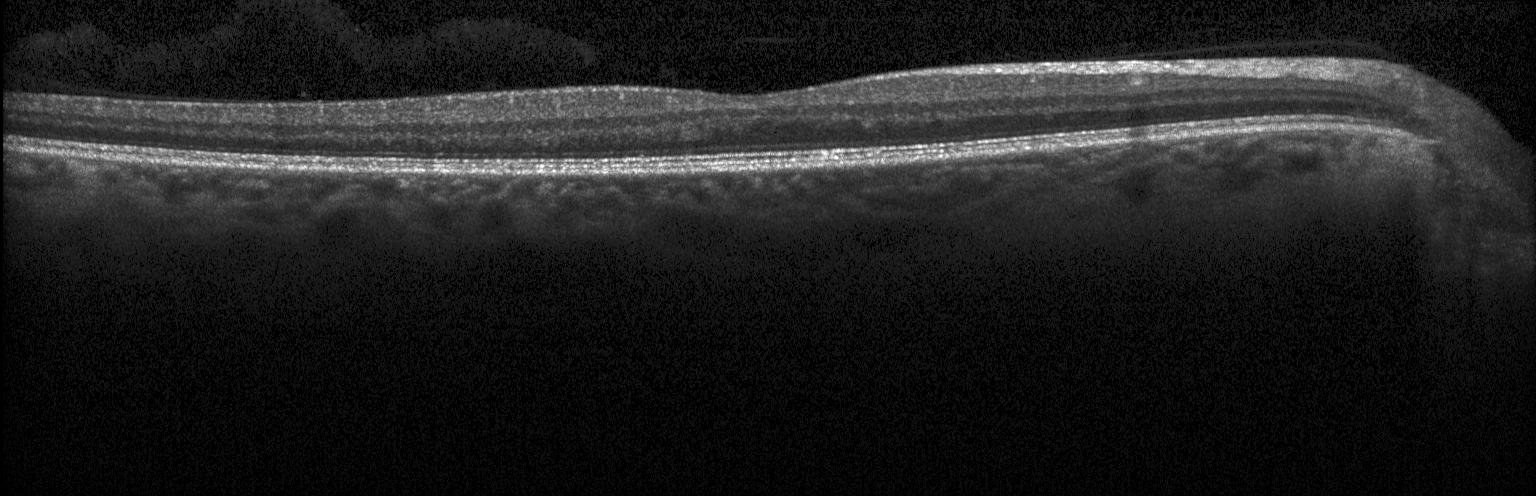

Heidelberg Spectralis OCT system; OCT line scan
Dx: no choroidal neovascularization, no diabetic macular edema, and no drusen.